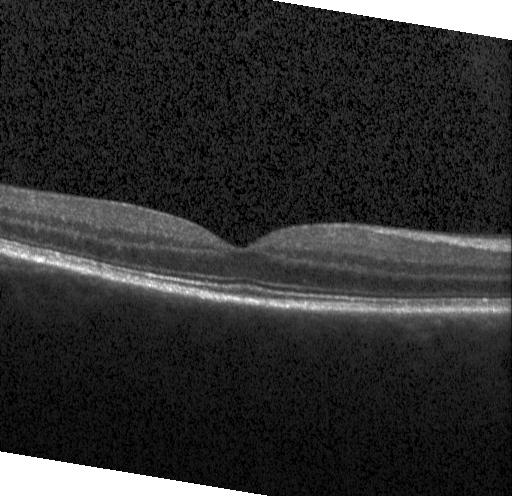
Diagnosis: no choroidal neovascularization, no diabetic macular edema, and no drusen.